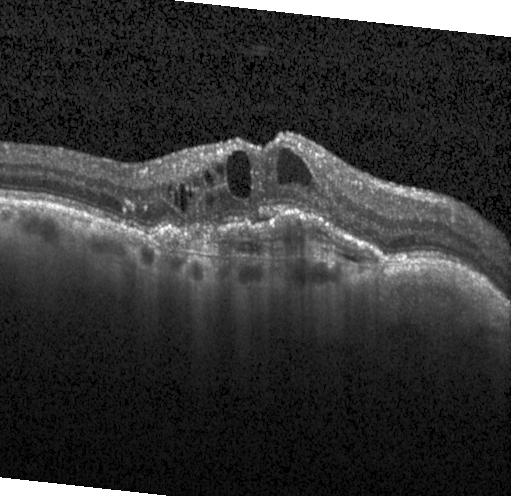 SD-OCT · fovea-centered · Heidelberg Spectralis · OCT line scan. A choroidal neovascular membrane.